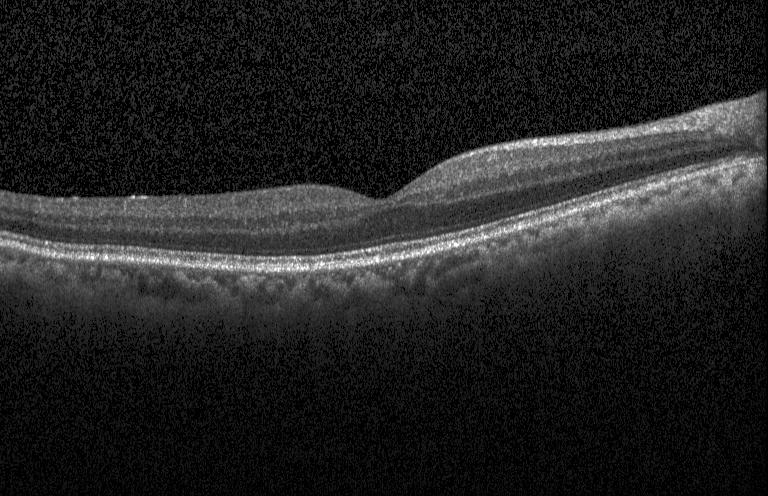
Impression: no choroidal neovascularization, no diabetic macular edema, and no drusen.